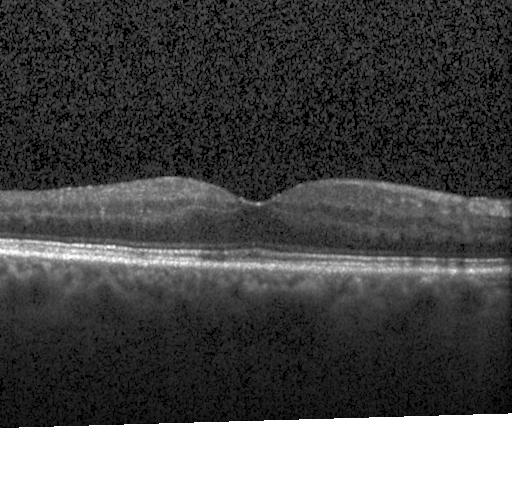
Optical coherence tomography B-scan.
Finding: neither choroidal neovascularization, diabetic macular edema, nor drusen.